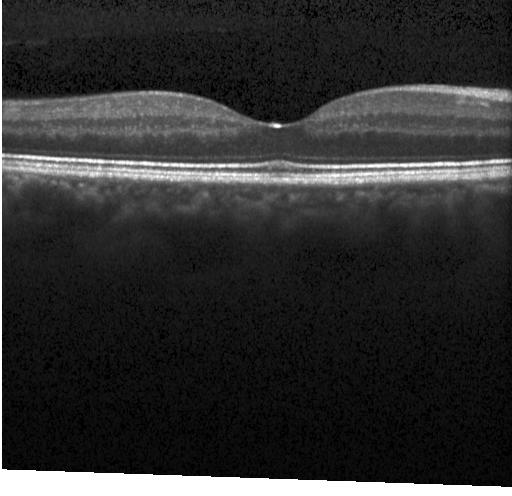
Dx: no evidence of choroidal neovascularization, diabetic macular edema, or drusen.